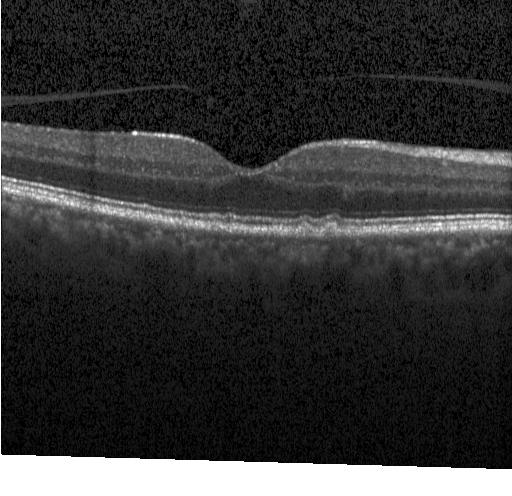 Through the macula · Heidelberg Spectralis OCT system · OCT B-scan — The scan shows multiple drusen.